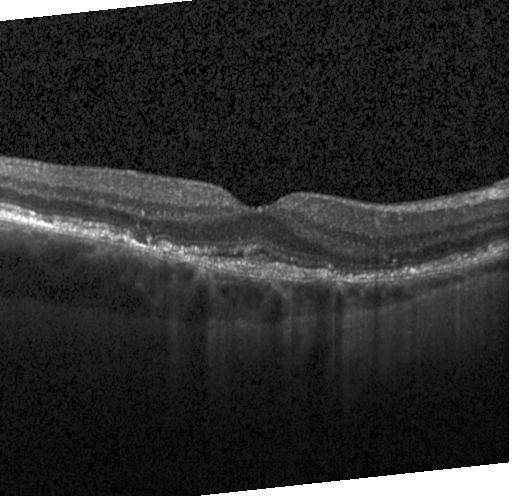
Diagnosis: a choroidal neovascular membrane.